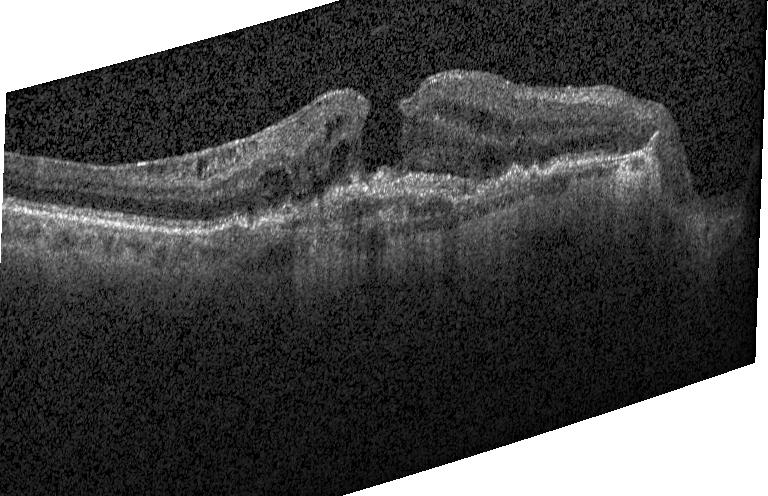 Acquired on a Heidelberg Spectralis; retinal OCT cross-section — Diagnosis: choroidal neovascularization (CNV).